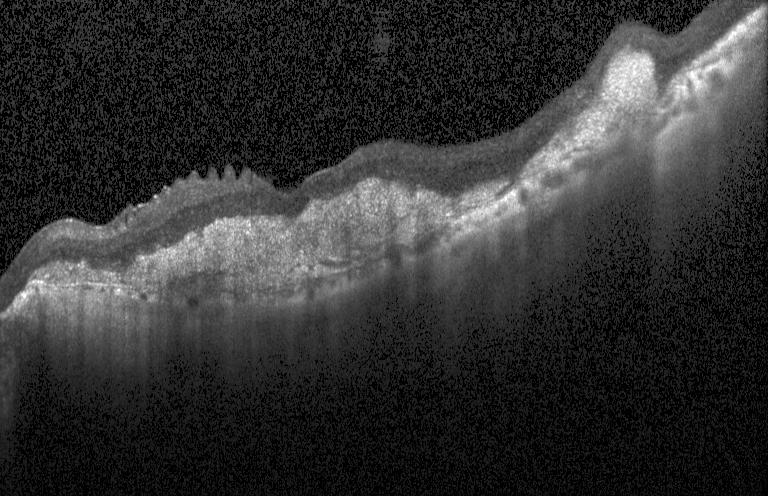

Retinal OCT cross-section showing a choroidal neovascular membrane.